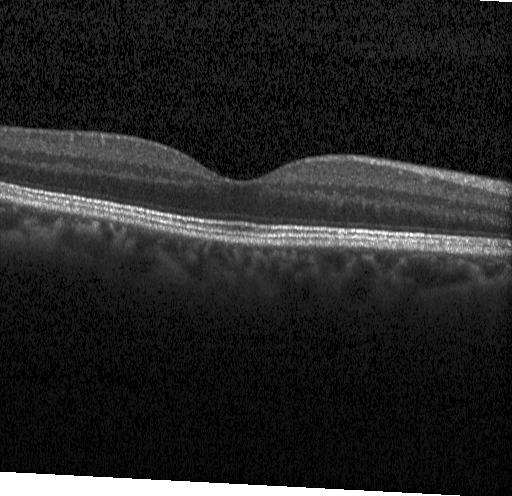 Diagnosis: neither choroidal neovascularization, diabetic macular edema, nor drusen.